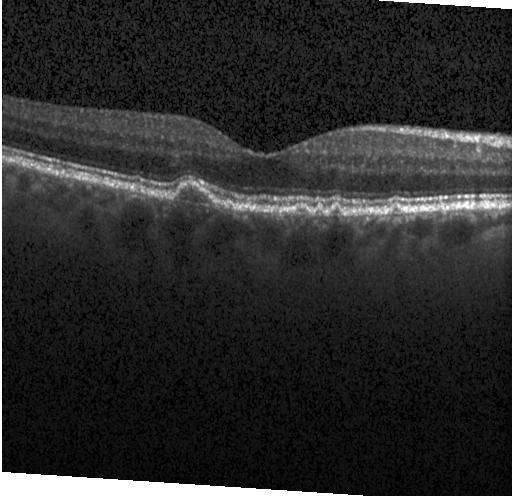 Retinal OCT cross-section showing multiple drusen.